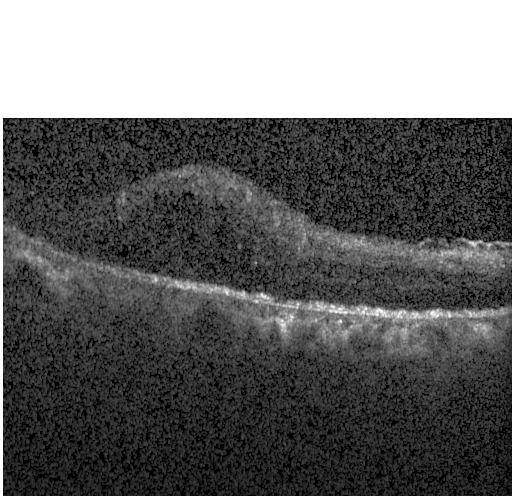

Horizontal scan through the fovea; SD-OCT; OCT line scan
This B-scan demonstrates diabetic macular edema.